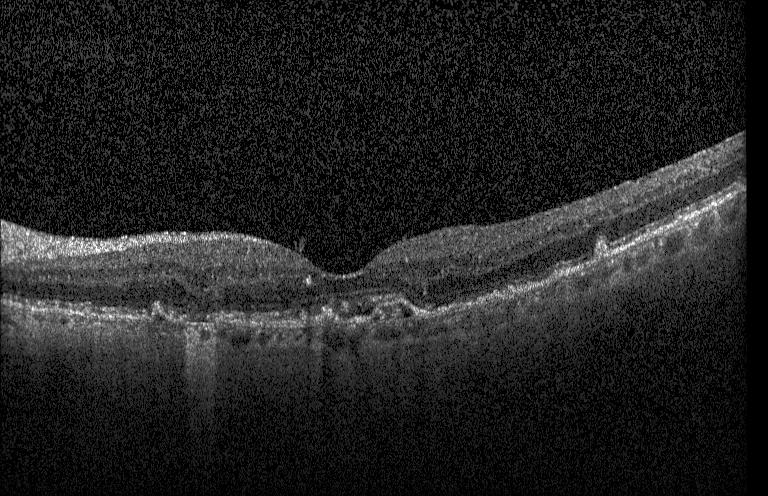
Horizontal scan through the fovea. Retinal OCT B-scan. Spectral-domain OCT. Acquired on a Heidelberg Spectralis. Diagnosis: choroidal neovascularization (CNV).